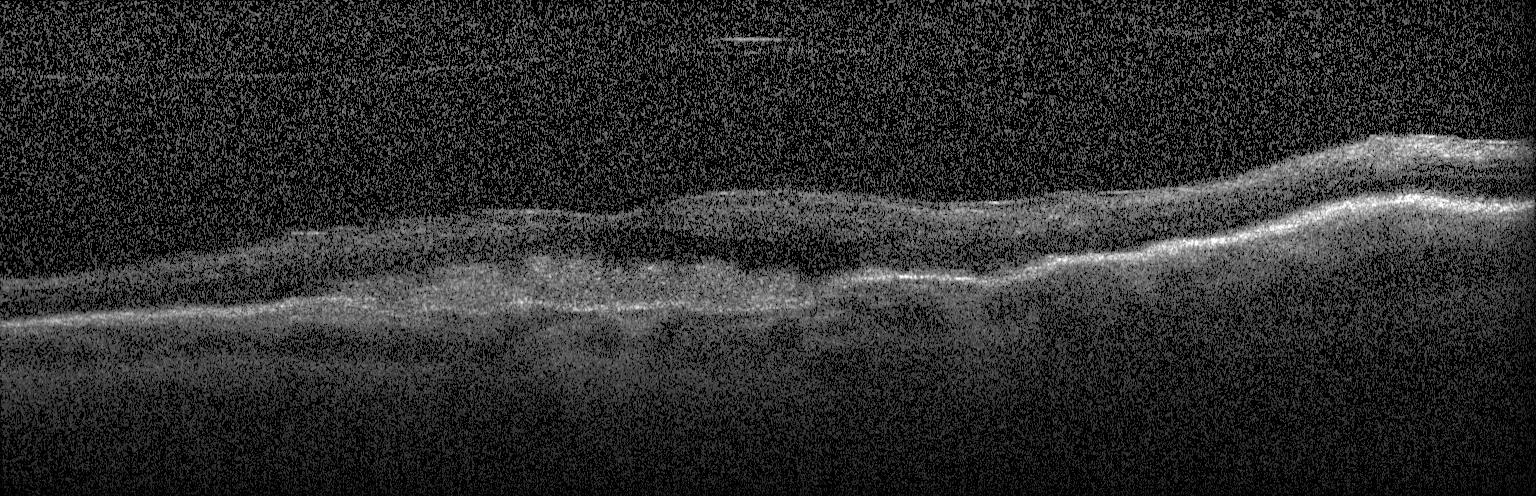 OCT scan showing a choroidal neovascular membrane.